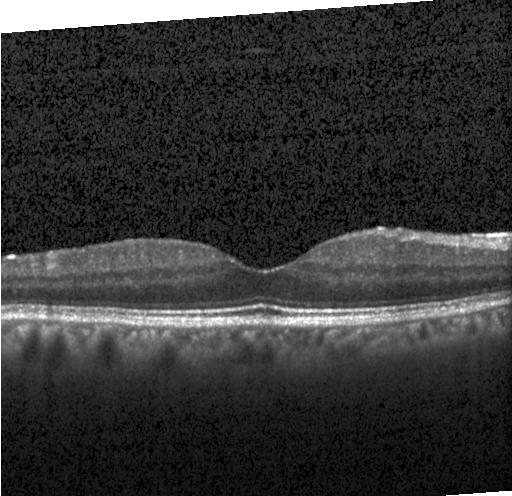 Heidelberg Spectralis. Optical coherence tomography B-scan. Impression: no choroidal neovascularization, no diabetic macular edema, and no drusen.